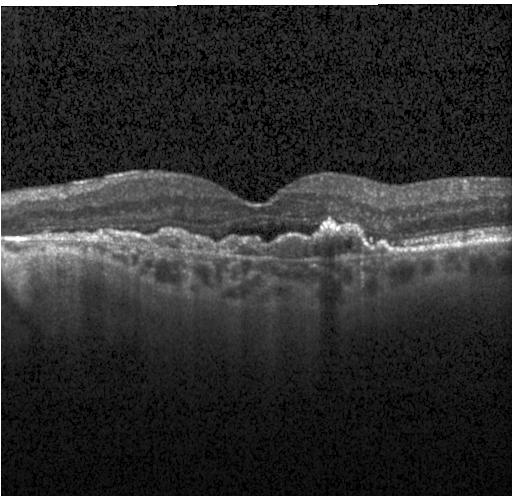

Horizontal scan through the fovea. Spectral-domain OCT. OCT line scan. Heidelberg Spectralis — OCT finding: a choroidal neovascular membrane.